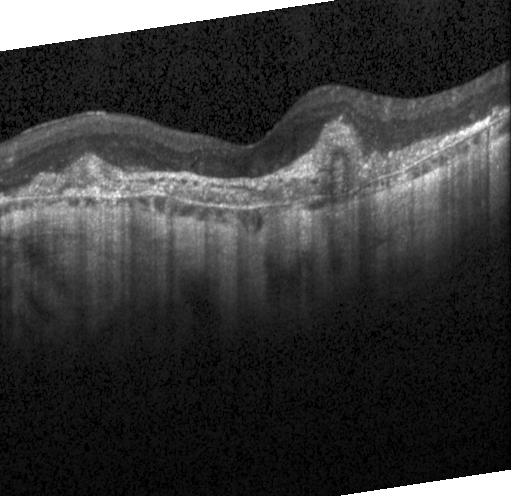

Spectral-domain OCT · Heidelberg Spectralis OCT system · optical coherence tomography scan.
Finding: a choroidal neovascular membrane.